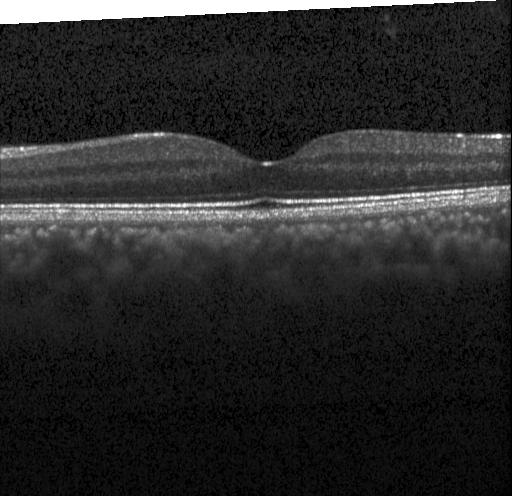

Diagnosis: neither choroidal neovascularization, diabetic macular edema, nor drusen.